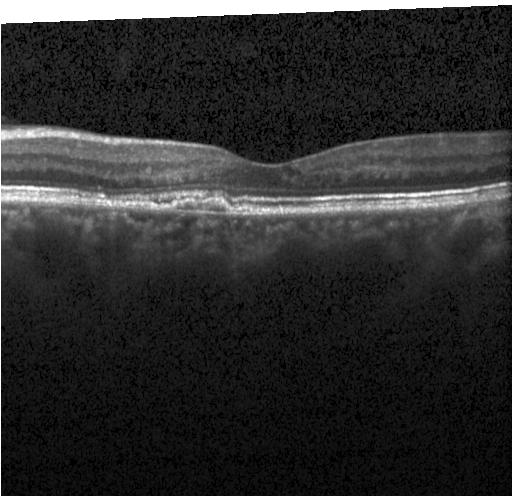 Through the macula, spectral-domain OCT, retinal OCT B-scan, acquired on a Heidelberg Spectralis. Finding: CNV.